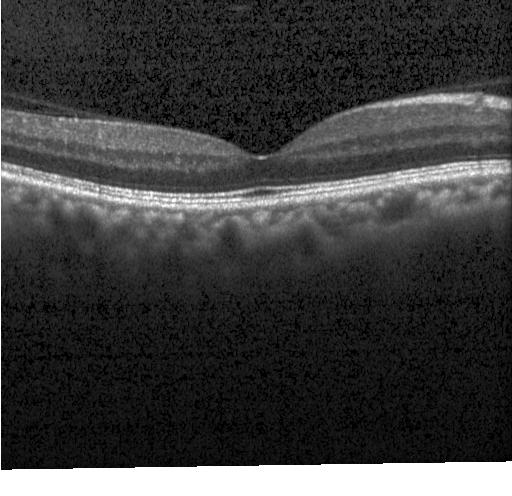
Dx: no choroidal neovascularization, no diabetic macular edema, and no drusen.